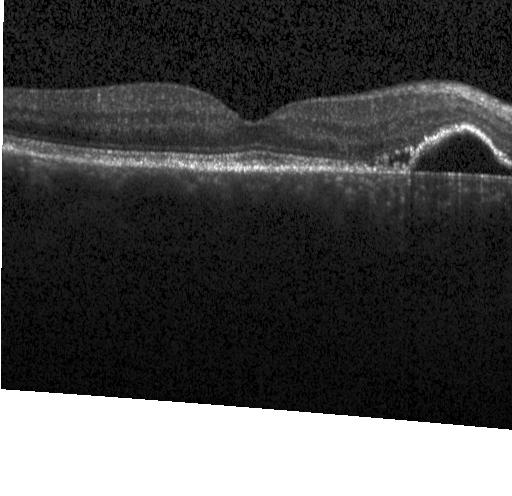 OCT finding: CNV.